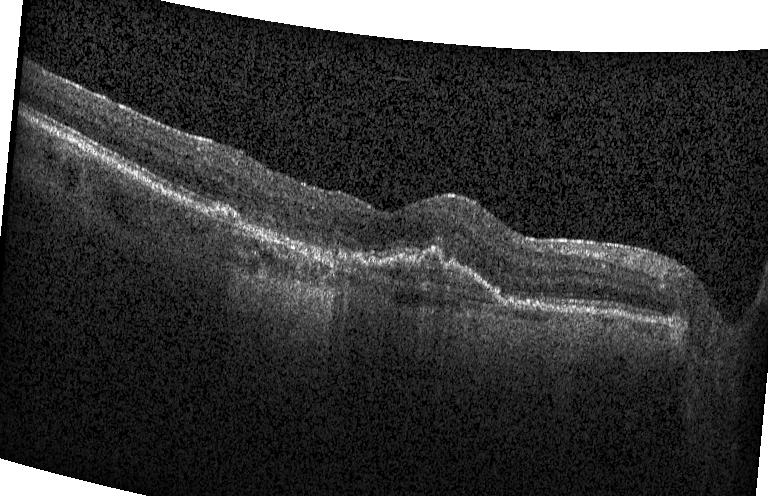

Centered on the fovea. Optical coherence tomography scan.
Finding: choroidal neovascularization (CNV).